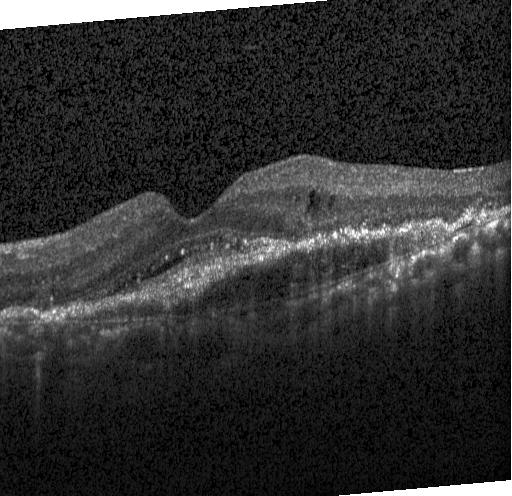
OCT B-scan.
Assessment: a choroidal neovascular membrane.